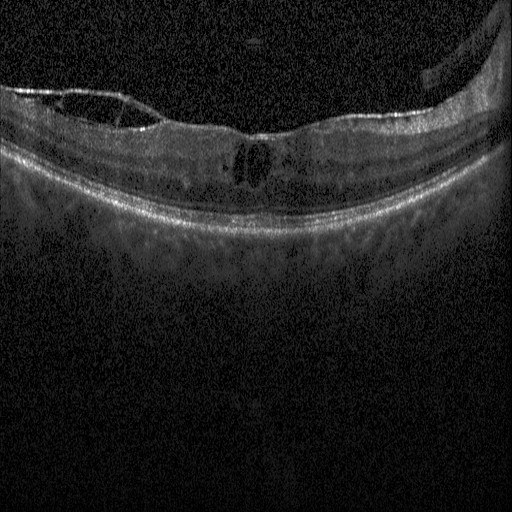

Retinal OCT B-scan; fovea-centered; Heidelberg Spectralis; spectral-domain optical coherence tomography. Finding: diabetic macular edema (DME).